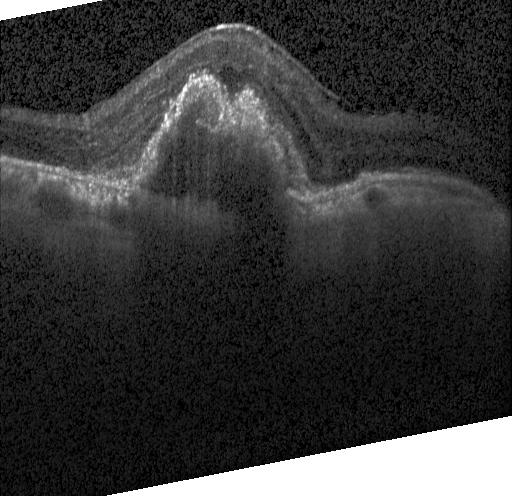
Macular OCT: choroidal neovascularization.